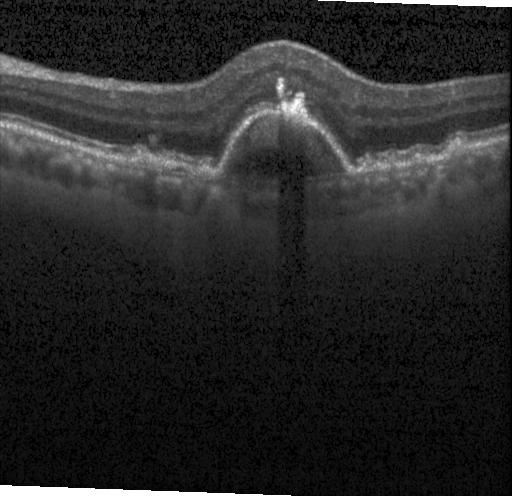
This B-scan demonstrates multiple drusen.